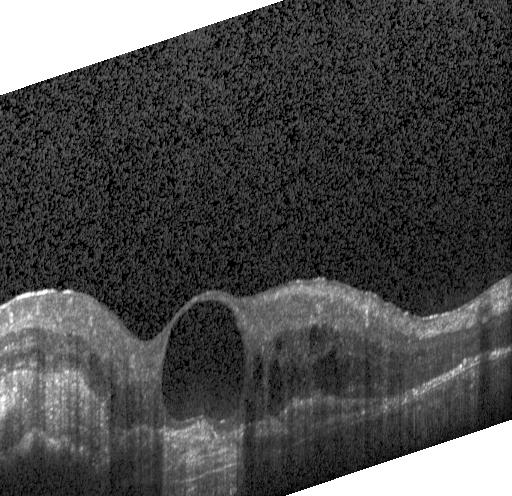

Optical coherence tomography scan. Centered on the fovea. Spectral-domain optical coherence tomography. Heidelberg Spectralis.
Macular OCT: CNV.